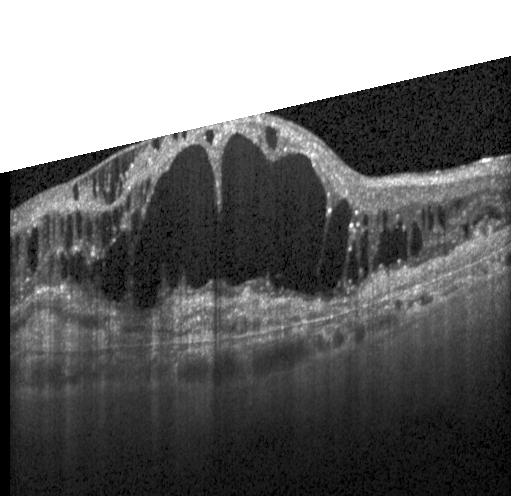
OCT line scan
Impression: a choroidal neovascular membrane.